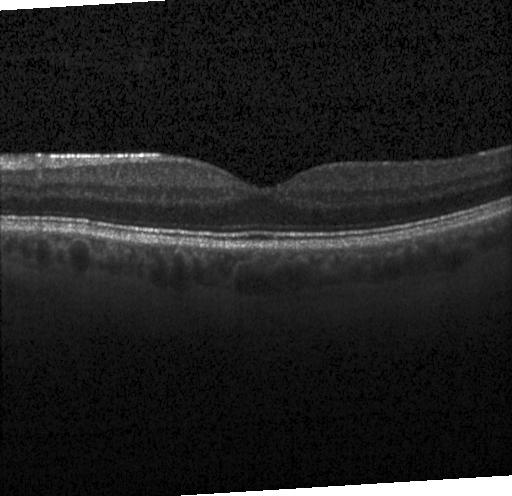
Macular OCT: neither choroidal neovascularization, diabetic macular edema, nor drusen.